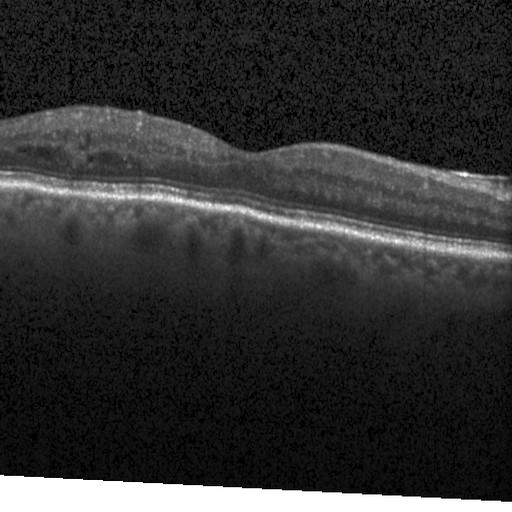
Retinal OCT B-scan. Diagnosis: diabetic macular edema.